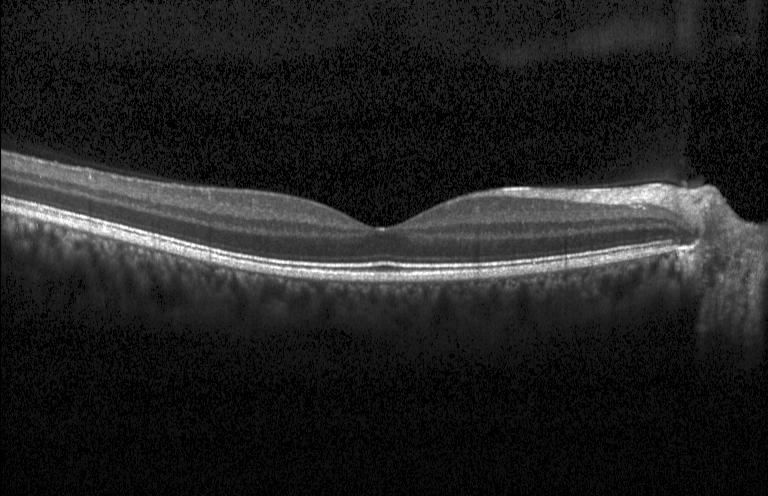

Impression: no evidence of choroidal neovascularization, diabetic macular edema, or drusen.